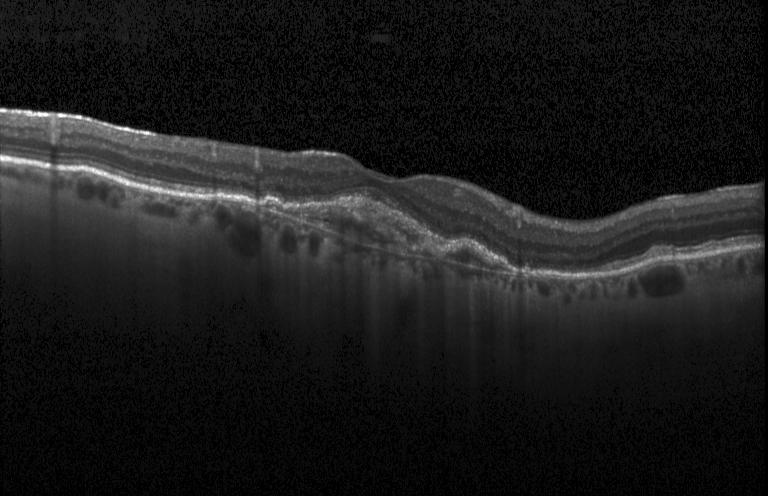
Macular scan; optical coherence tomography scan. A choroidal neovascular membrane.